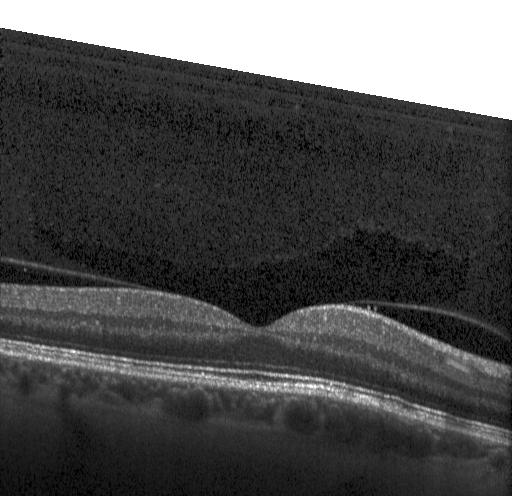

This B-scan demonstrates neither CNV, DME, nor drusen.